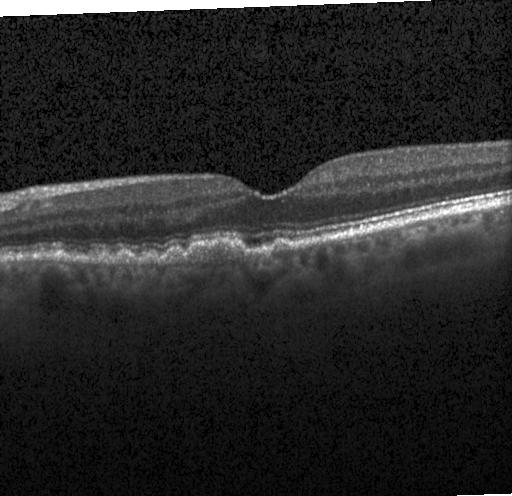

Optical coherence tomography scan.
Impression: sub-RPE drusenoid deposits.